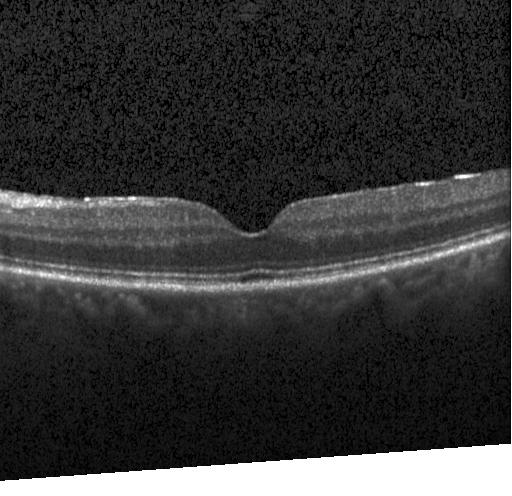 Optical coherence tomography scan — Impression: no evidence of choroidal neovascularization, diabetic macular edema, or drusen.